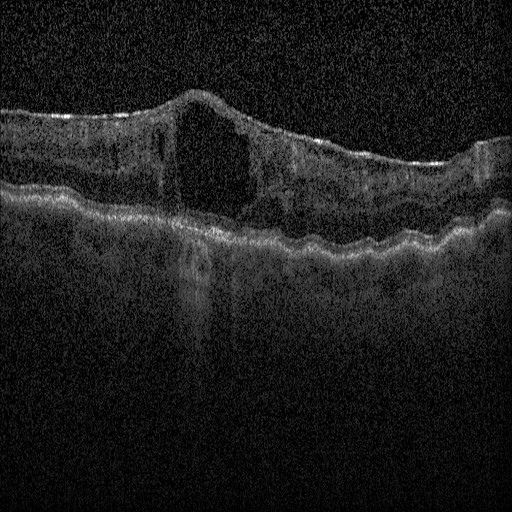 Fovea-centered · optical coherence tomography scan
Finding: diabetic macular edema (DME).